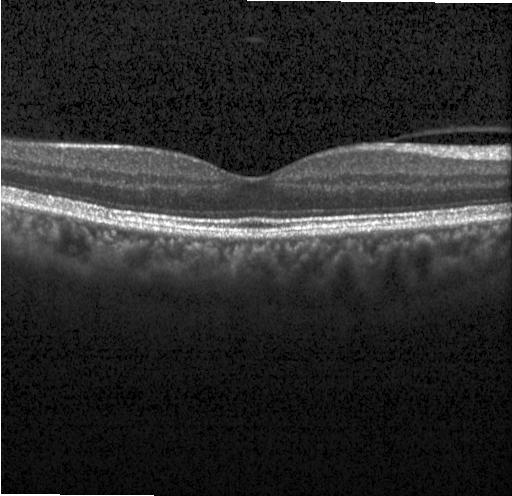
OCT finding: neither choroidal neovascularization, diabetic macular edema, nor drusen.